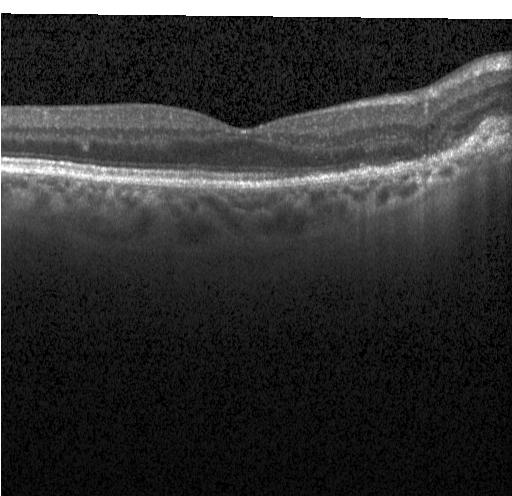
OCT line scan · centered on the fovea · acquired on a Heidelberg Spectralis · spectral-domain optical coherence tomography. Diagnosis: a choroidal neovascular membrane.